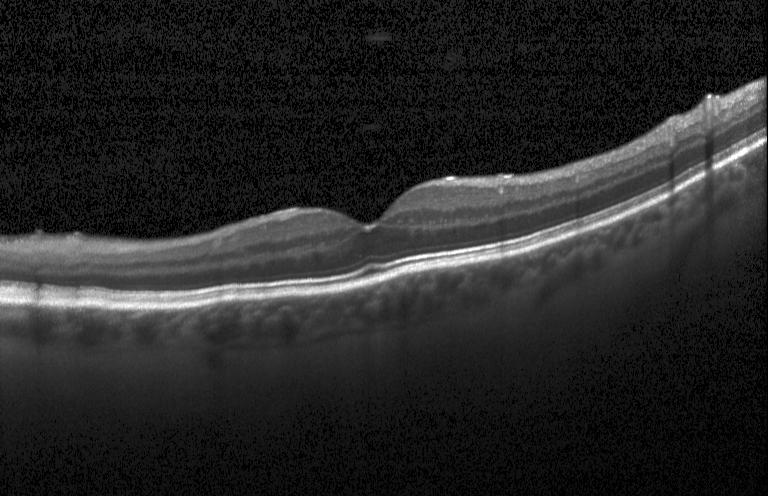

Through the macula, retinal OCT cross-section. This B-scan demonstrates no evidence of CNV, DME, or drusen.